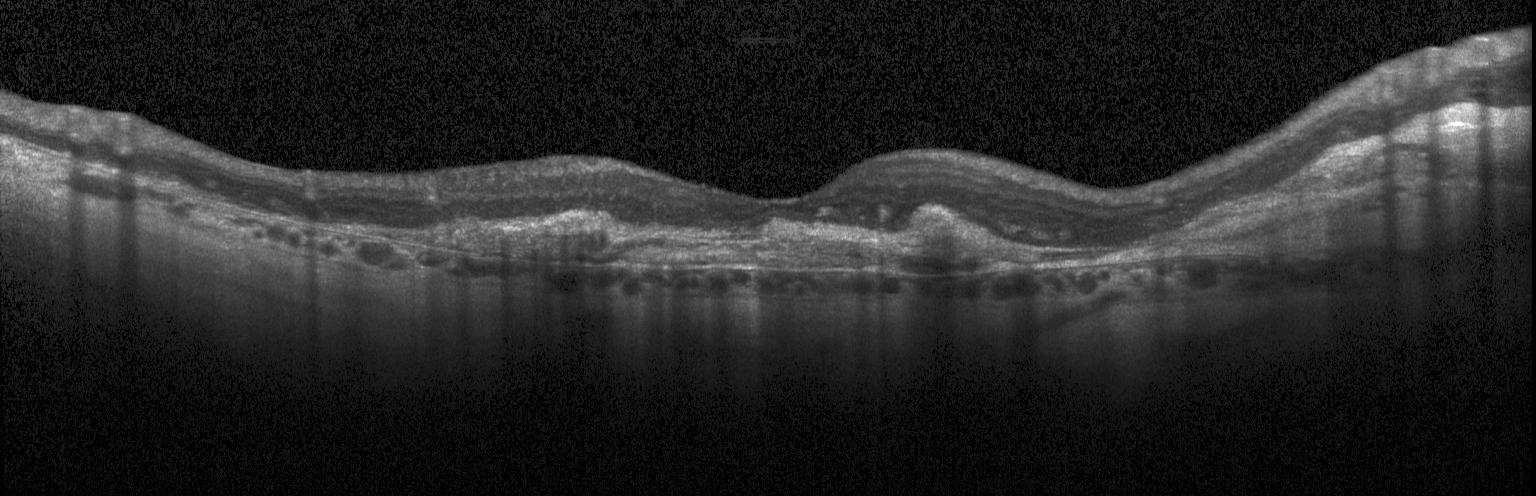
OCT B-scan. Impression: a choroidal neovascular membrane.